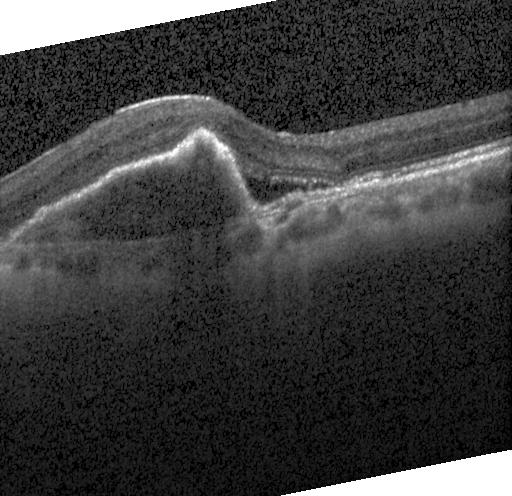 Fovea-centered; SD-OCT; retinal OCT B-scan; Heidelberg Spectralis. Impression: a choroidal neovascular membrane.